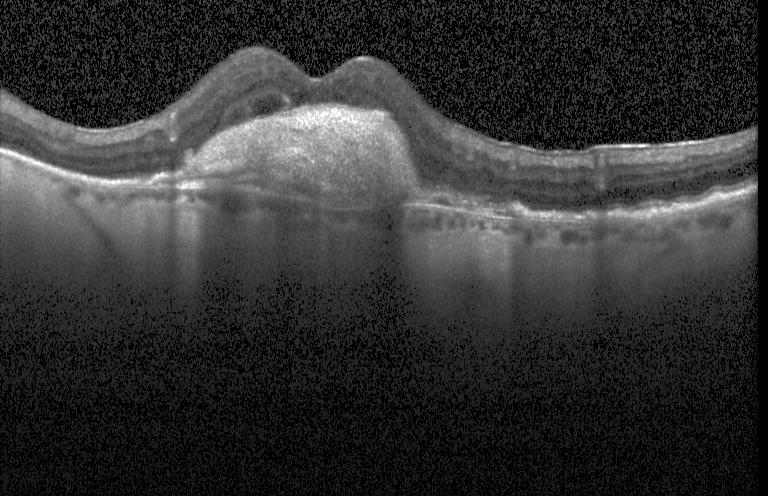

Optical coherence tomography B-scan
The scan shows CNV.